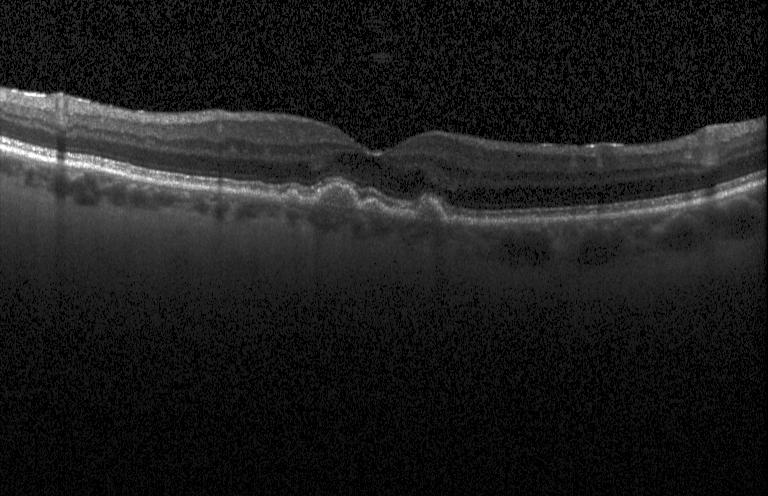

OCT line scan.
This B-scan demonstrates sub-RPE drusenoid deposits.